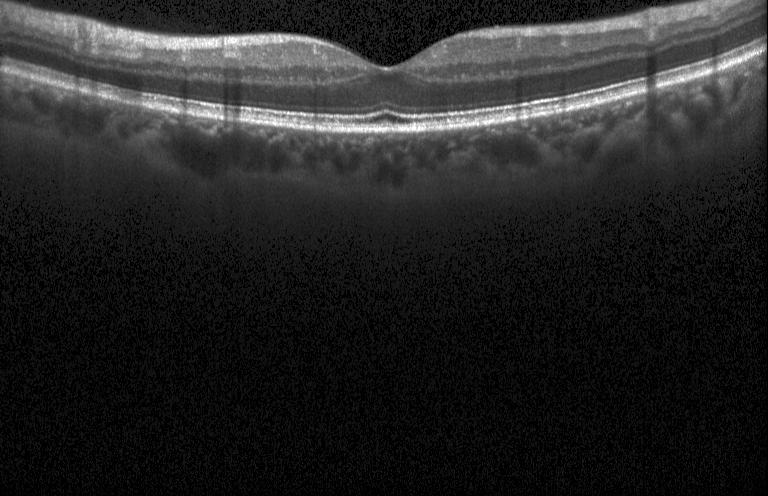
Assessment: no evidence of choroidal neovascularization, diabetic macular edema, or drusen.